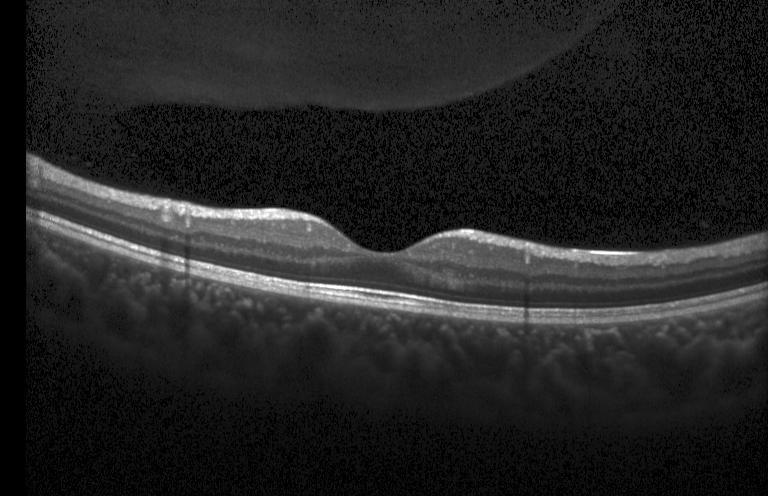 Macular OCT: neither choroidal neovascularization, diabetic macular edema, nor drusen.